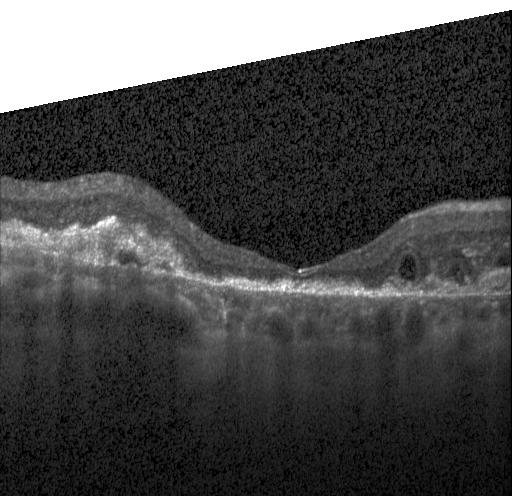
Retinal OCT cross-section · SD-OCT.
Choroidal neovascularization.